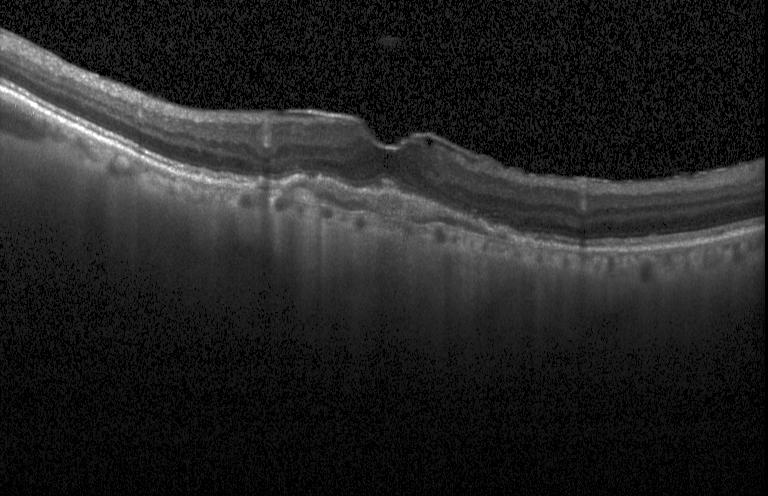

Diagnosis: a choroidal neovascular membrane.